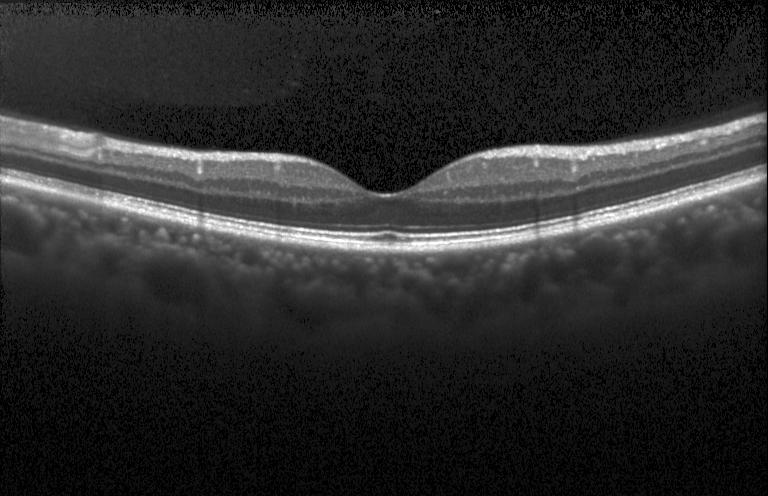
The scan shows no choroidal neovascularization, no diabetic macular edema, and no drusen.